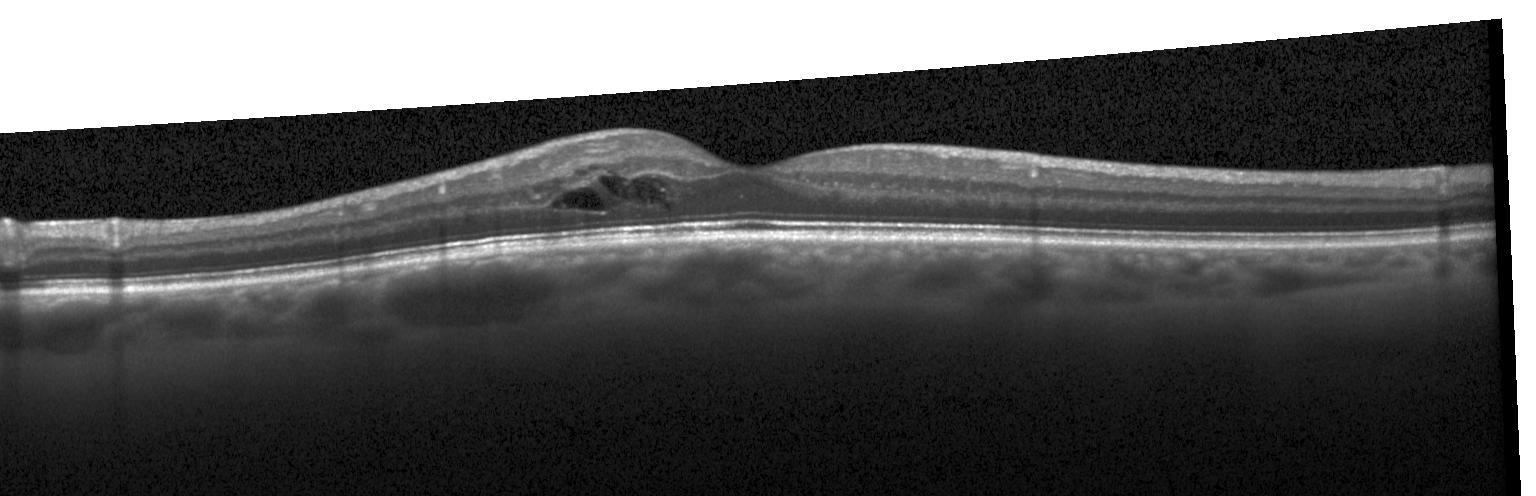
OCT B-scan showing diabetic macular edema.